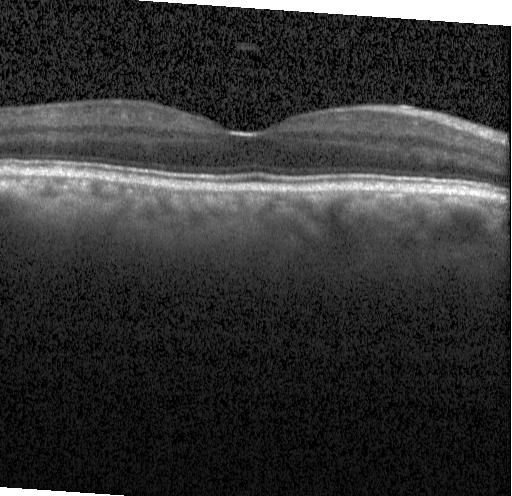 OCT line scan; instrument: Heidelberg Spectralis
Finding: neither CNV, DME, nor drusen.